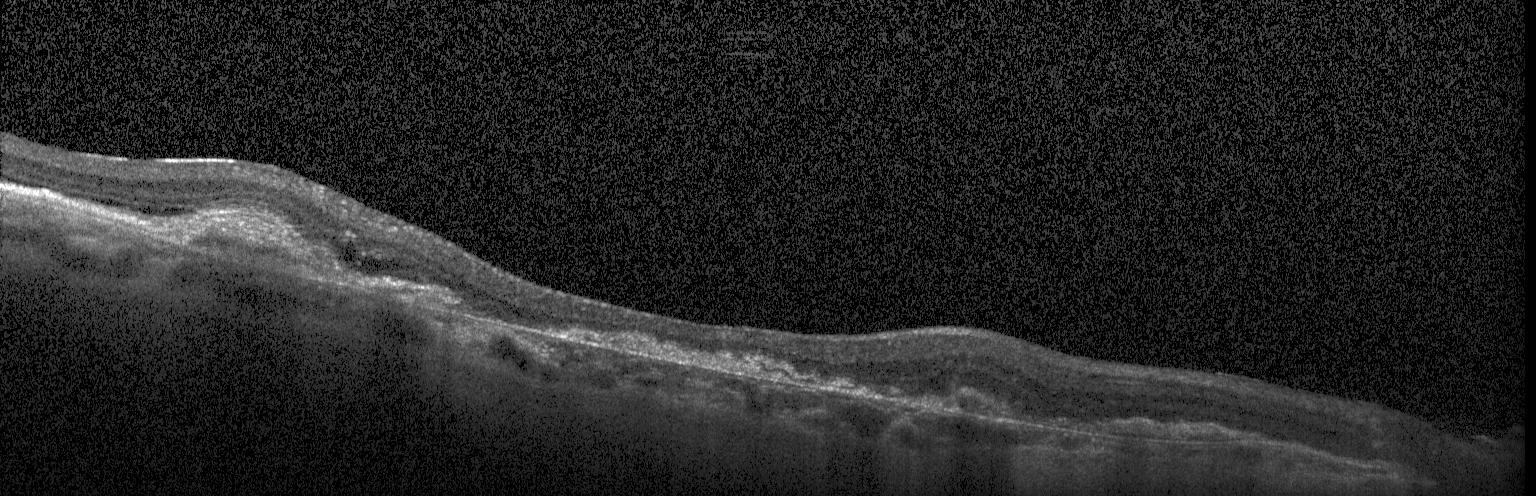 Fovea-centered, Heidelberg Spectralis OCT system, OCT B-scan. Impression: a choroidal neovascular membrane.